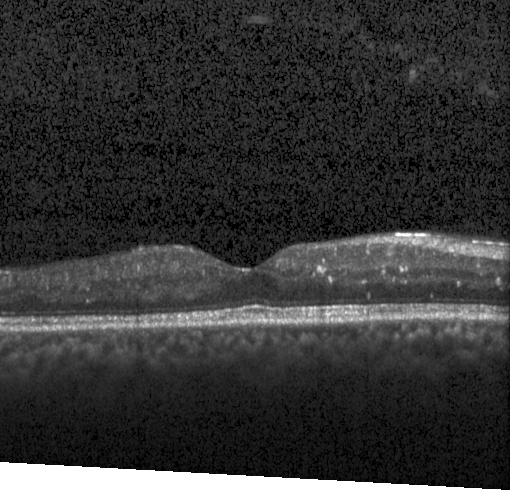 Spectral-domain optical coherence tomography. Retinal OCT cross-section
This B-scan demonstrates diabetic macular edema (DME).